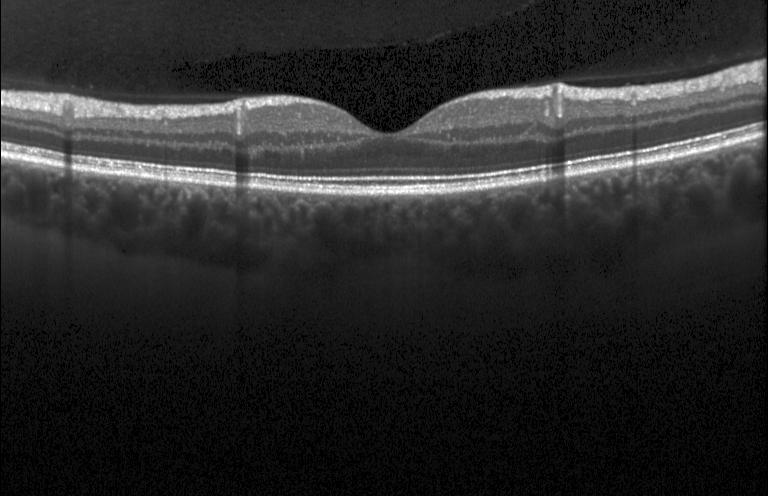

Centered on the fovea; SD-OCT; optical coherence tomography B-scan; Heidelberg Spectralis OCT system.
Dx: no evidence of CNV, DME, or drusen.